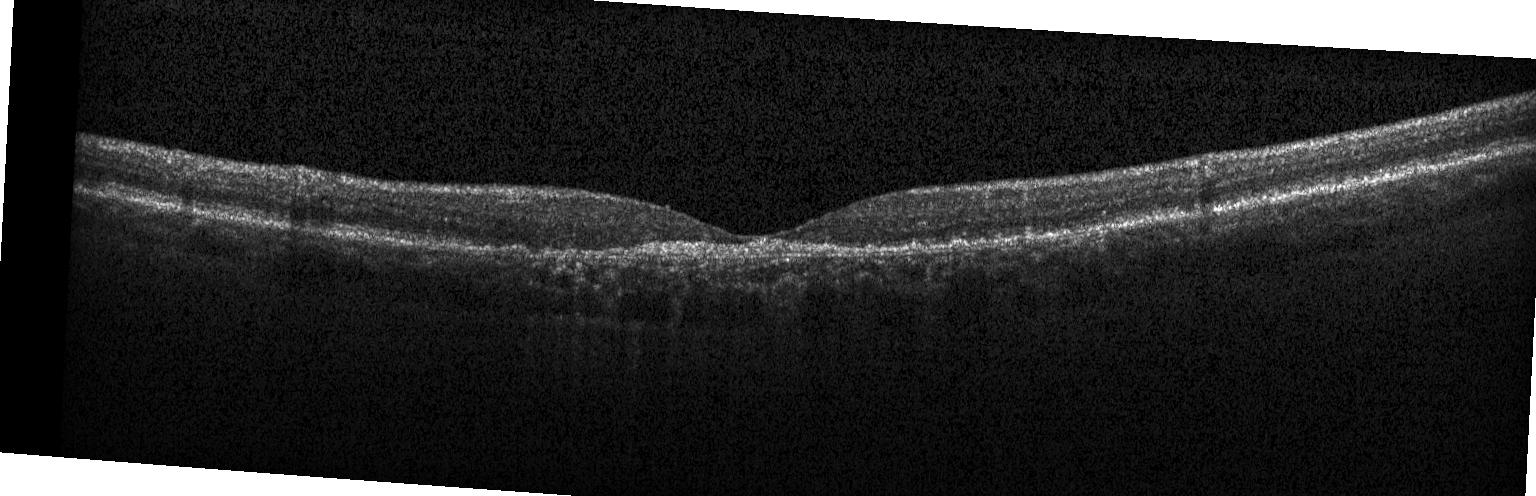
Finding: choroidal neovascularization (CNV).